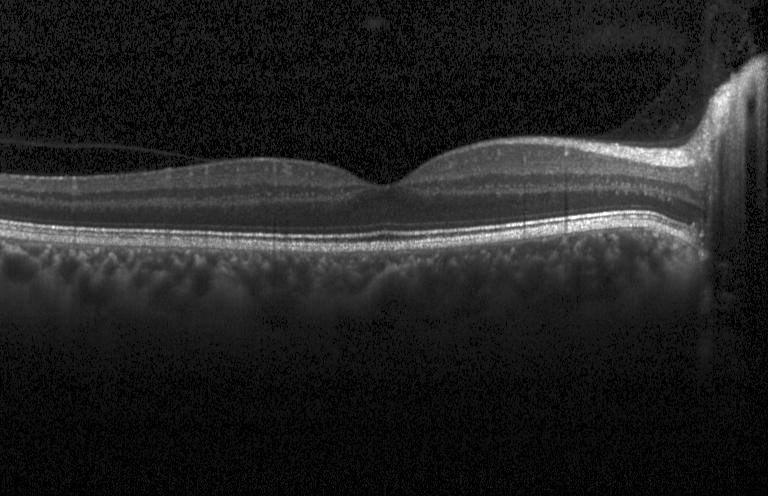 OCT line scan, spectral-domain OCT, fovea-centered, instrument: Heidelberg Spectralis — OCT finding: neither choroidal neovascularization, diabetic macular edema, nor drusen.